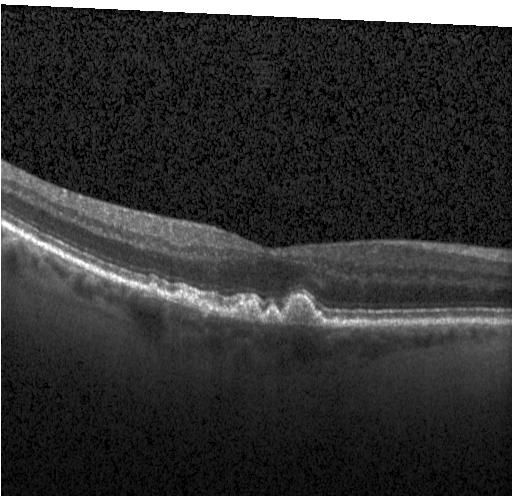

OCT line scan. Diagnosis: sub-RPE drusenoid deposits.